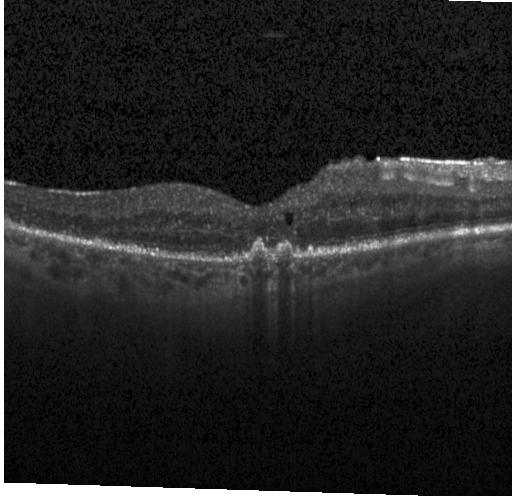 Diagnosis: a choroidal neovascular membrane.